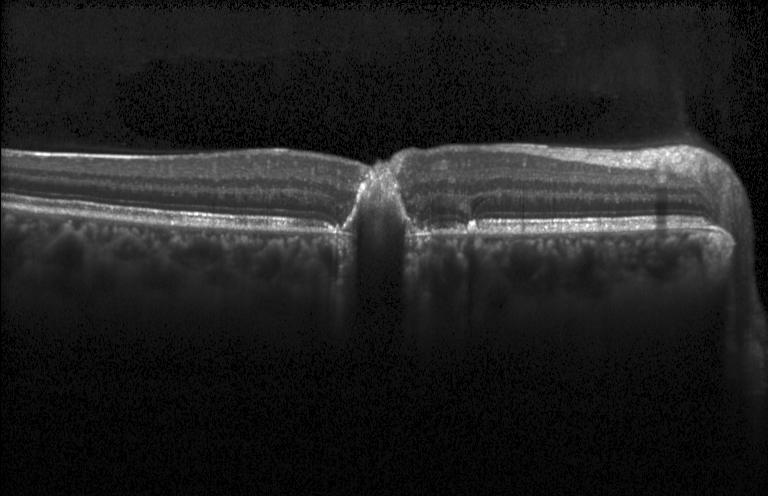
Retinal OCT cross-section showing choroidal neovascularization.